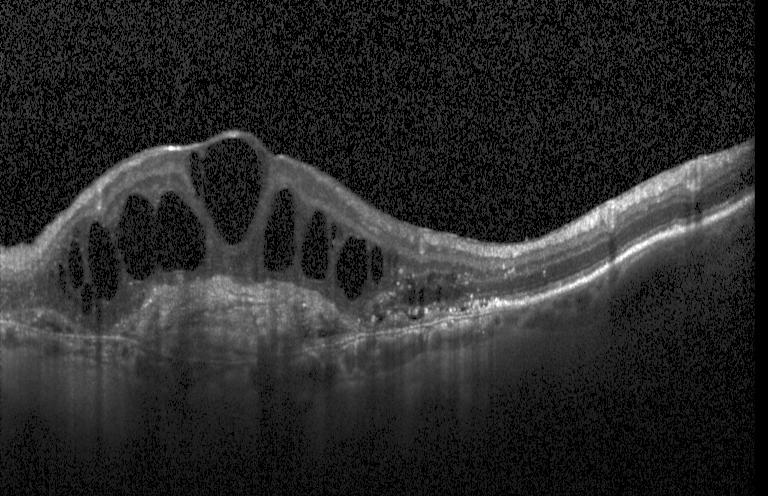 Optical coherence tomography scan. SD-OCT.
The scan shows a choroidal neovascular membrane.